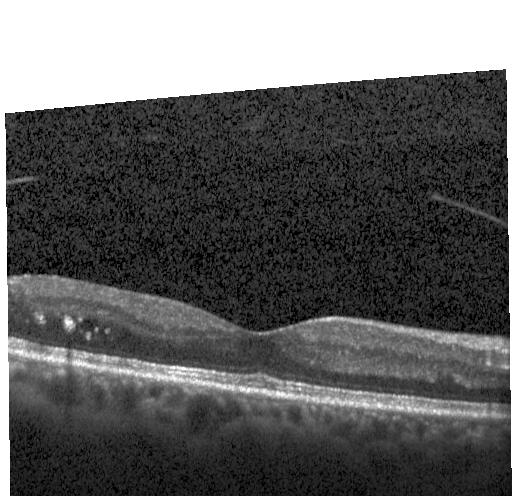
Optical coherence tomography B-scan
This B-scan demonstrates diabetic macular edema (DME).